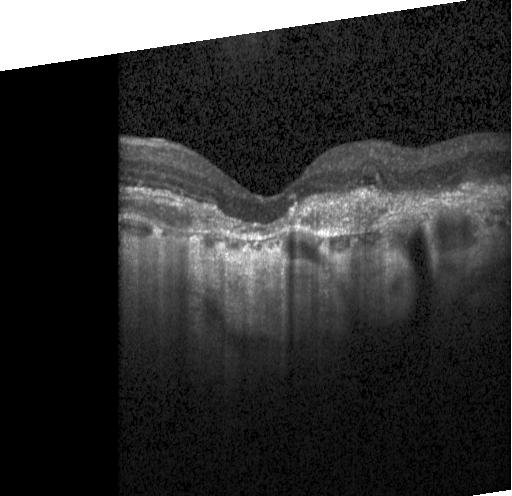 Acquired on a Heidelberg Spectralis, retinal OCT B-scan. Impression: choroidal neovascularization (CNV).